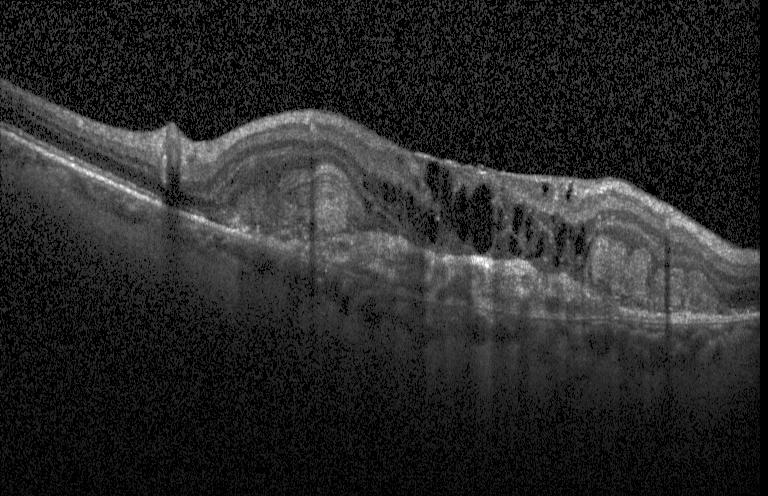 Impression: choroidal neovascularization (CNV).